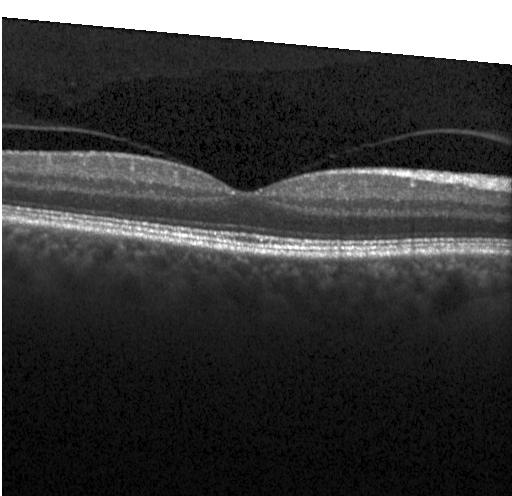 OCT line scan.
The scan shows no CNV, no DME, and no drusen.